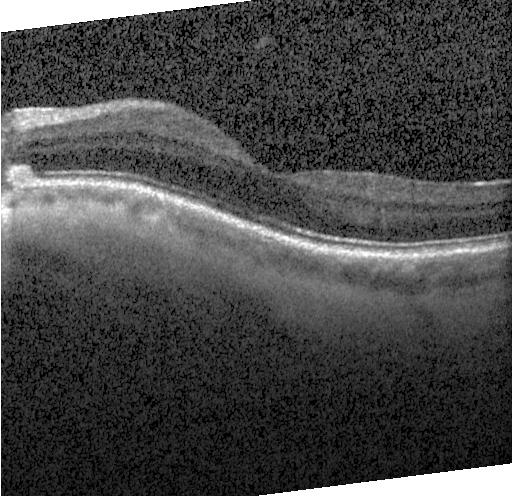

OCT B-scan
Macular OCT: drusen.